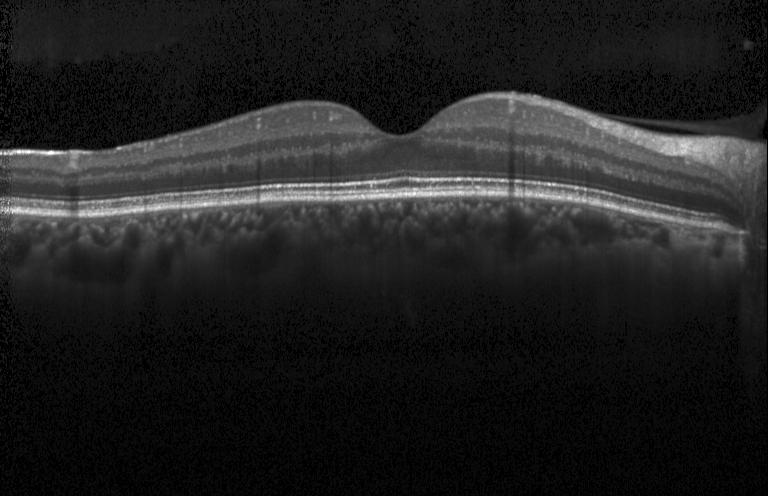 Optical coherence tomography scan
No choroidal neovascularization, diabetic macular edema, or drusen.